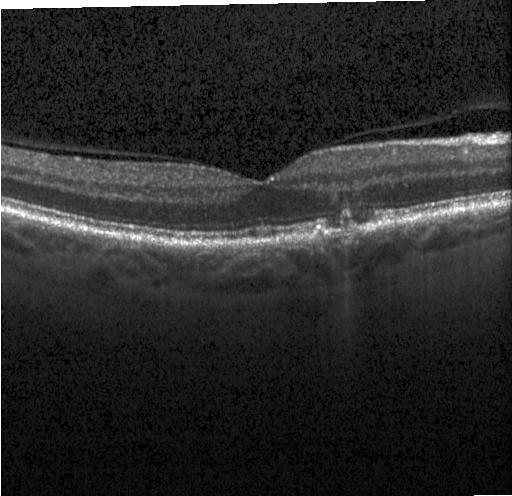
Retinal OCT cross-section, Heidelberg Spectralis — Macular OCT: sub-RPE drusenoid deposits.